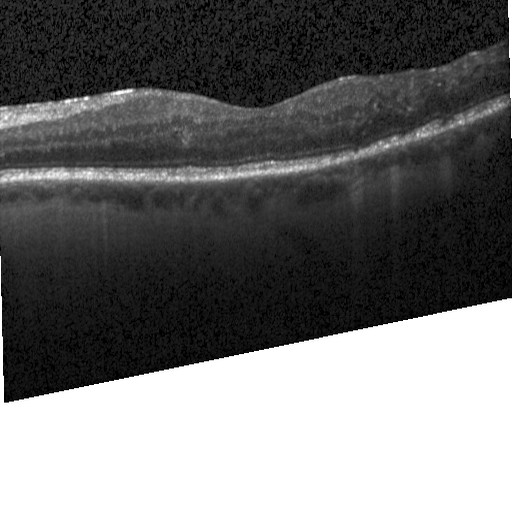
Finding: diabetic macular edema.